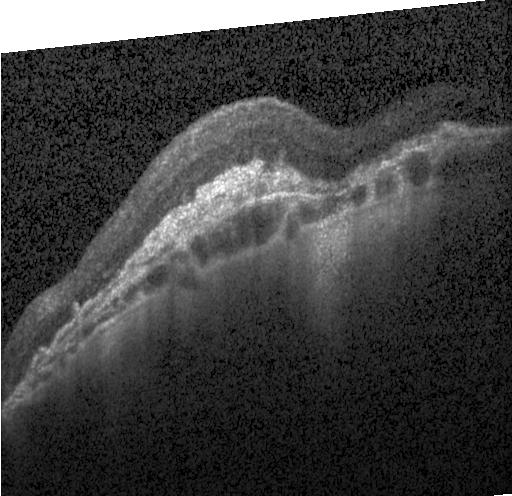 The scan shows CNV.